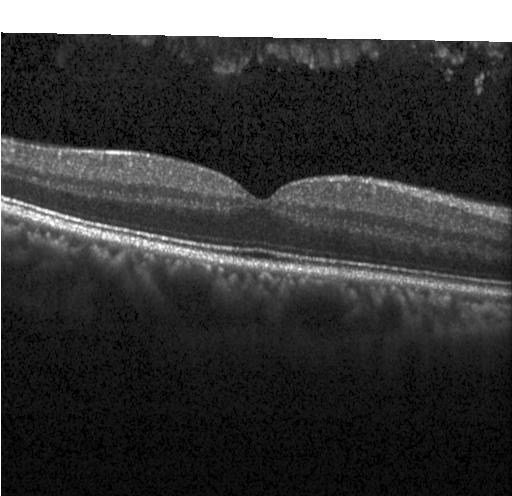 Macular scan. OCT B-scan. Spectral-domain OCT.
Diagnosis: no choroidal neovascularization, no diabetic macular edema, and no drusen.